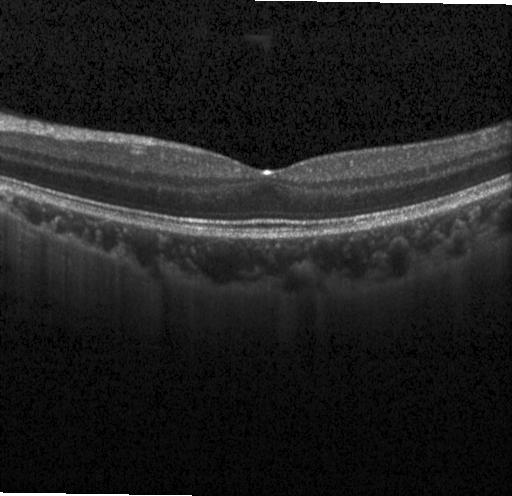 Horizontal scan through the fovea; optical coherence tomography B-scan; spectral-domain optical coherence tomography; Heidelberg Spectralis OCT system — This B-scan demonstrates no evidence of choroidal neovascularization, diabetic macular edema, or drusen.